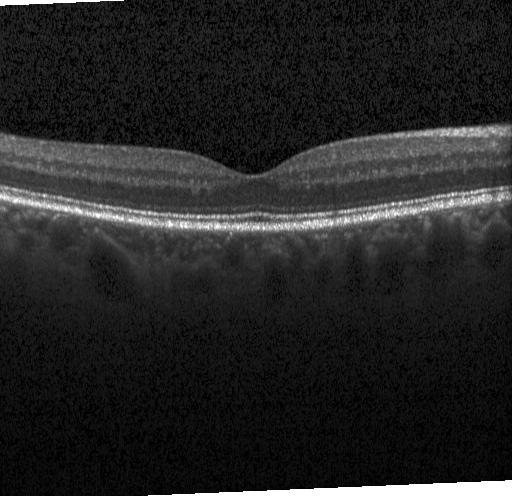
Optical coherence tomography B-scan · spectral-domain OCT · fovea-centered · Heidelberg Spectralis. Finding: neither CNV, DME, nor drusen.